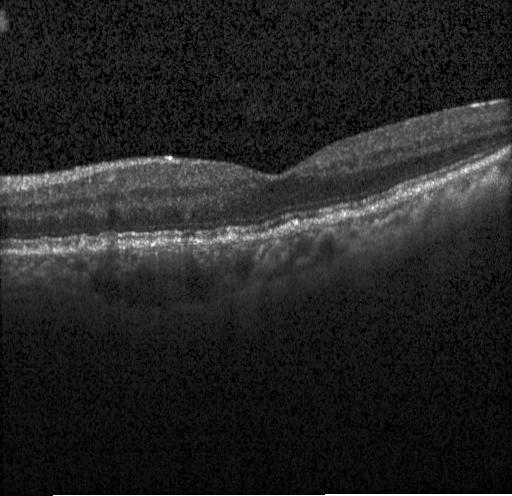

Finding: drusen.